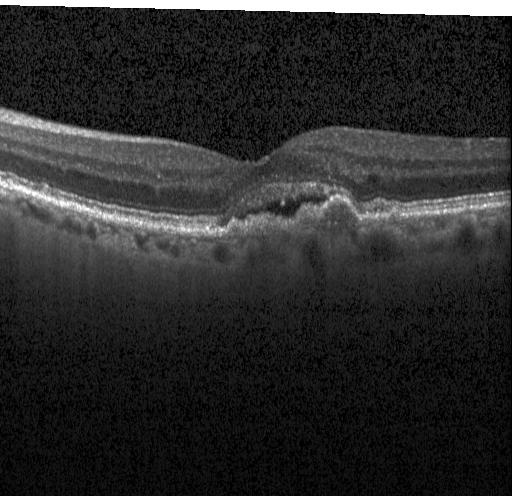 Centered on the fovea · OCT B-scan
Dx: a choroidal neovascular membrane.